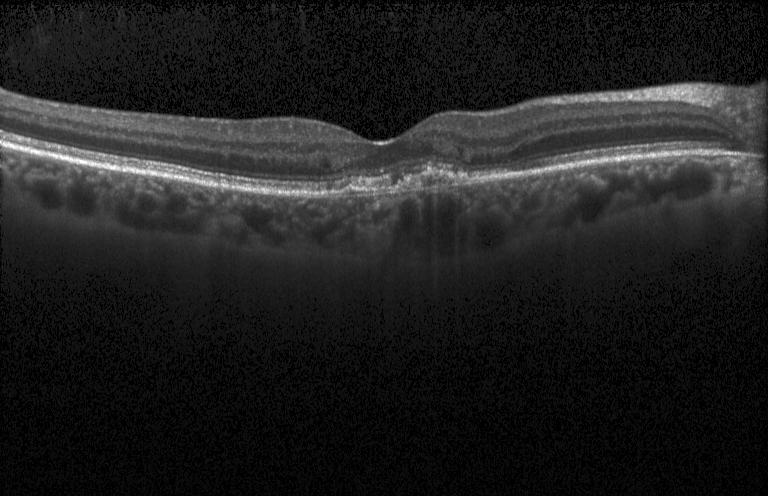
Optical coherence tomography B-scan. Heidelberg Spectralis OCT system. Spectral-domain optical coherence tomography. Dx: CNV.